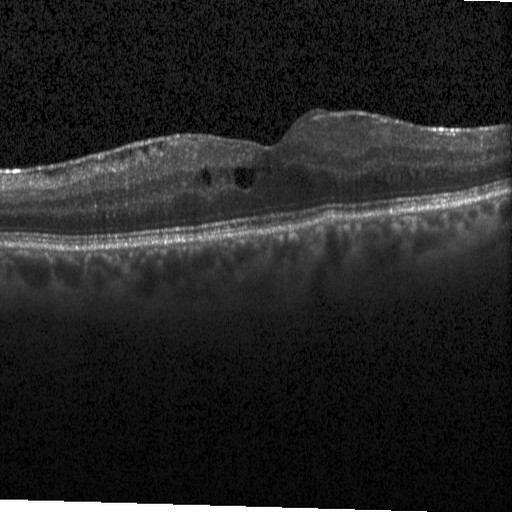

Optical coherence tomography B-scan. OCT finding: diabetic macular edema.